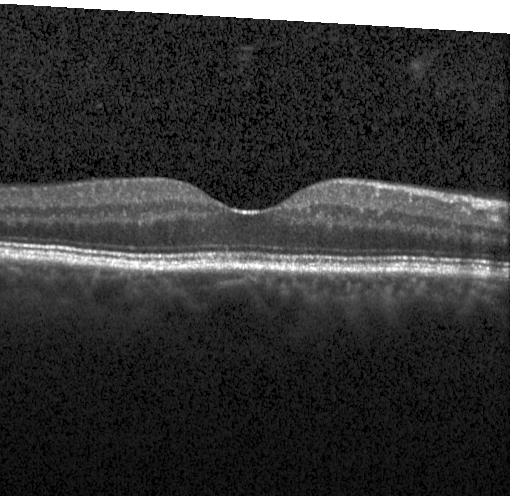

Macular OCT demonstrating no choroidal neovascularization, no diabetic macular edema, and no drusen.